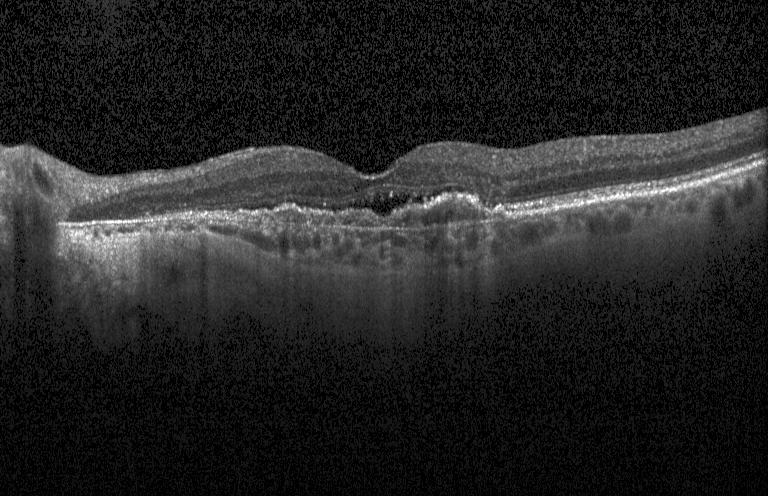 Heidelberg Spectralis OCT system · through the macula · spectral-domain optical coherence tomography · OCT line scan.
Finding: choroidal neovascularization.